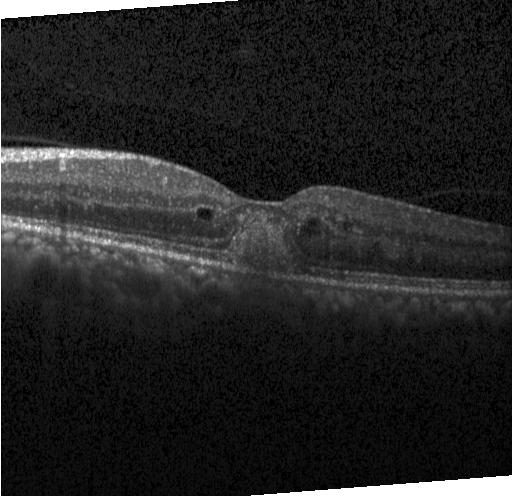
Retinal OCT cross-section; fovea-centered. The scan shows CNV.